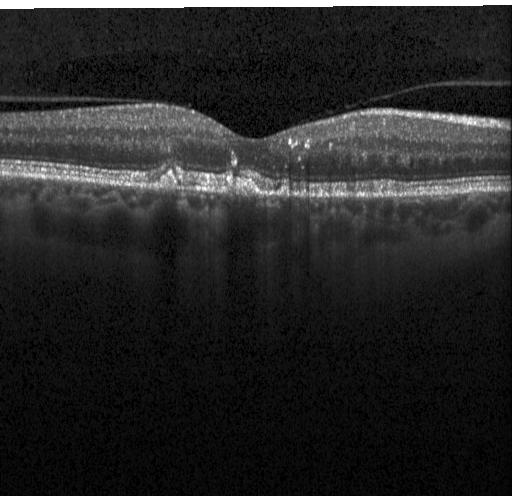

Heidelberg Spectralis OCT system · optical coherence tomography scan. Diagnosis: multiple drusen.